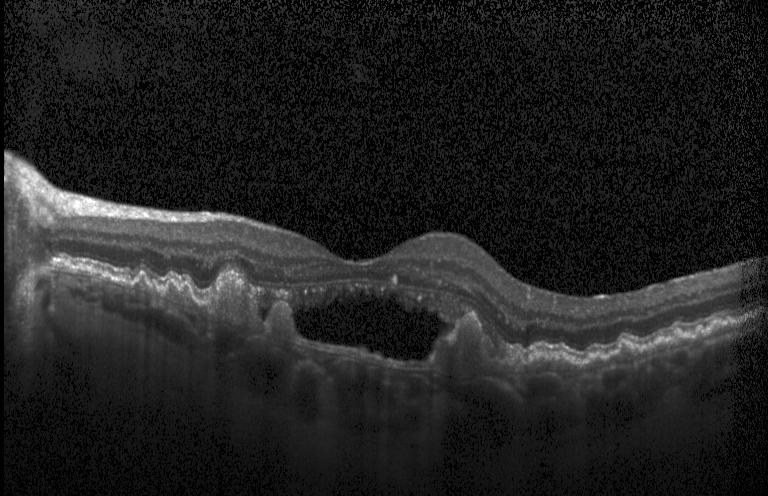

Heidelberg Spectralis OCT system; horizontal scan through the fovea; retinal OCT cross-section; SD-OCT. Finding: choroidal neovascularization.